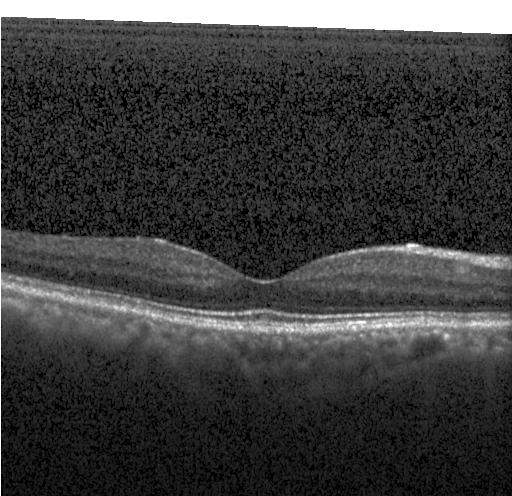

Spectral-domain optical coherence tomography. Centered on the fovea. Retinal OCT B-scan. Heidelberg Spectralis OCT system. Macular OCT: no evidence of choroidal neovascularization, diabetic macular edema, or drusen.